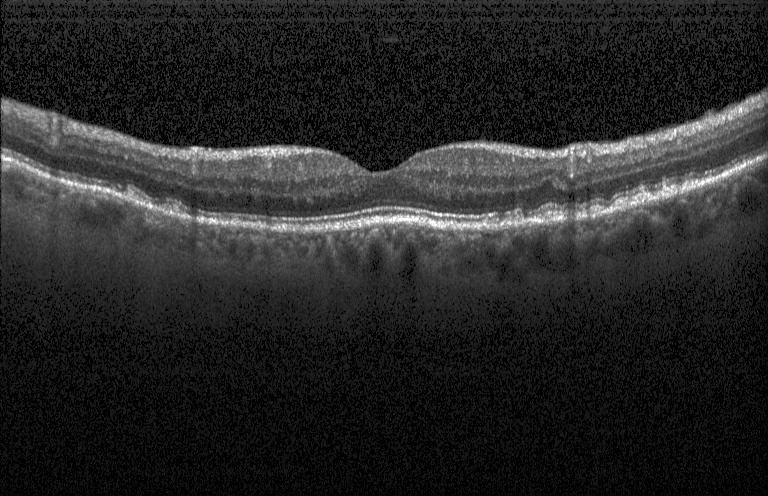 Multiple drusen.